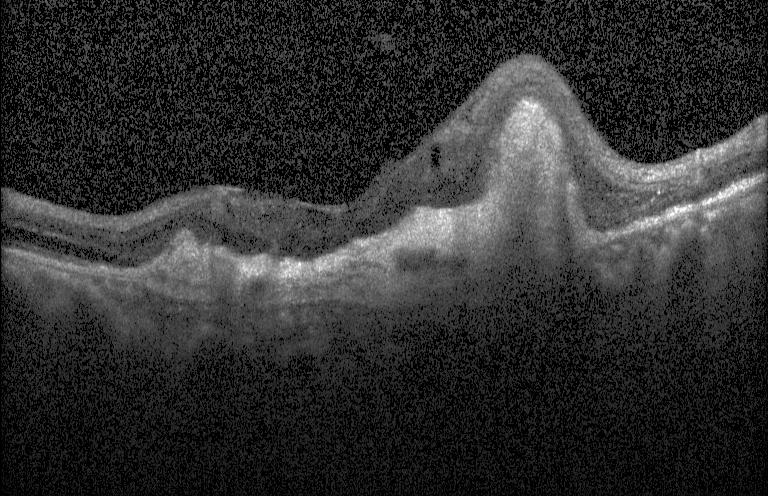 Optical coherence tomography B-scan; spectral-domain optical coherence tomography. This B-scan demonstrates choroidal neovascularization.